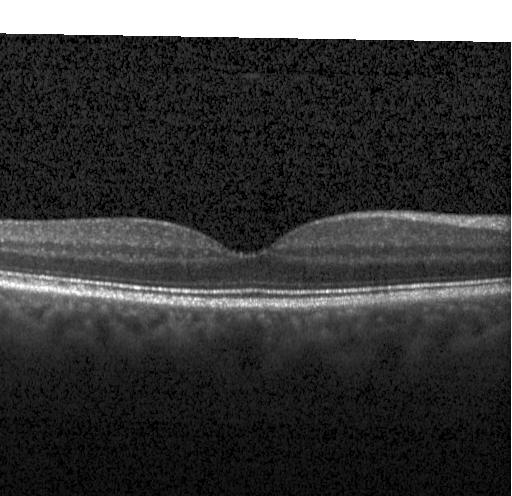

Retinal OCT cross-section · instrument: Heidelberg Spectralis — No evidence of choroidal neovascularization, diabetic macular edema, or drusen.